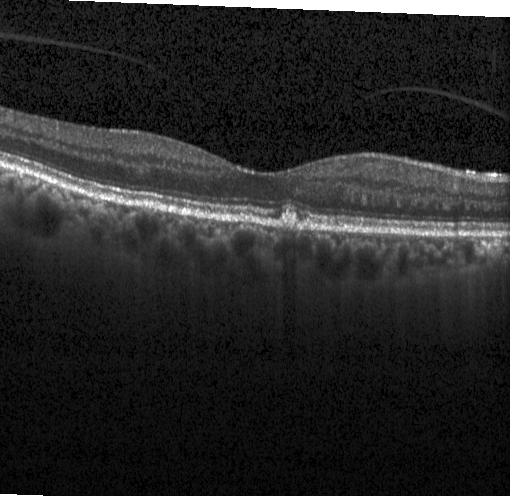 Macular OCT demonstrating multiple drusen.